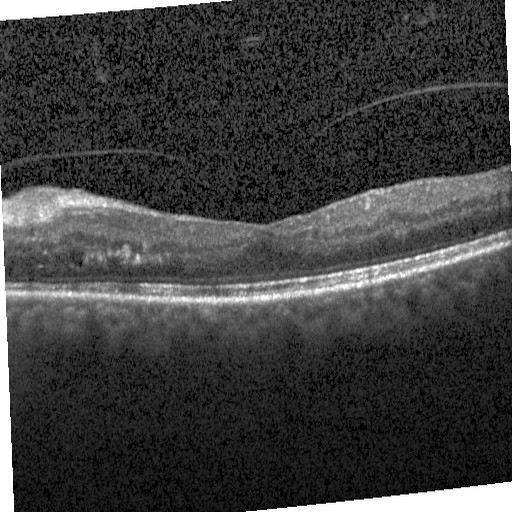 OCT B-scan showing diabetic macular edema.